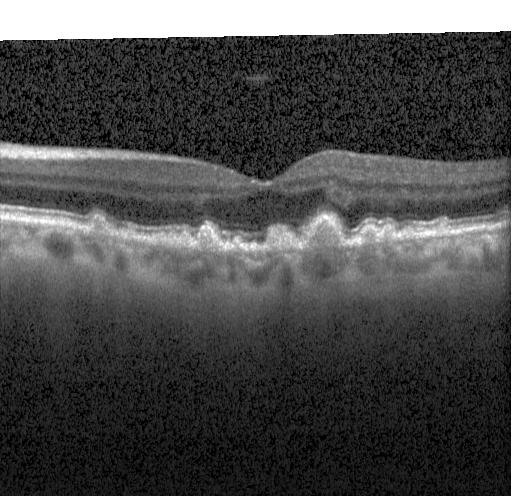
The scan shows drusen.